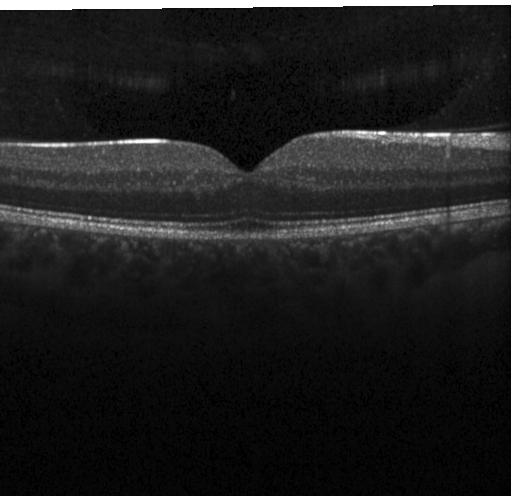
OCT finding: neither choroidal neovascularization, diabetic macular edema, nor drusen.